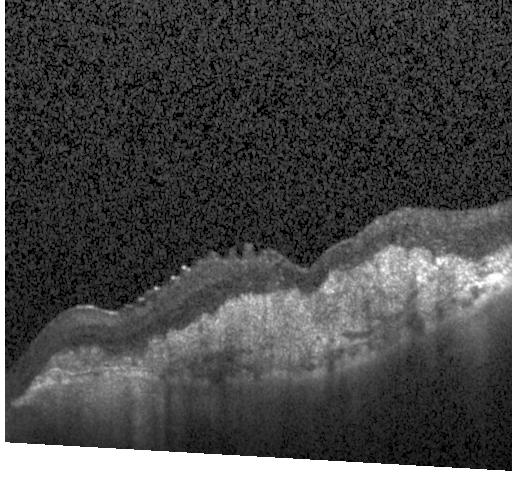
Finding: CNV.